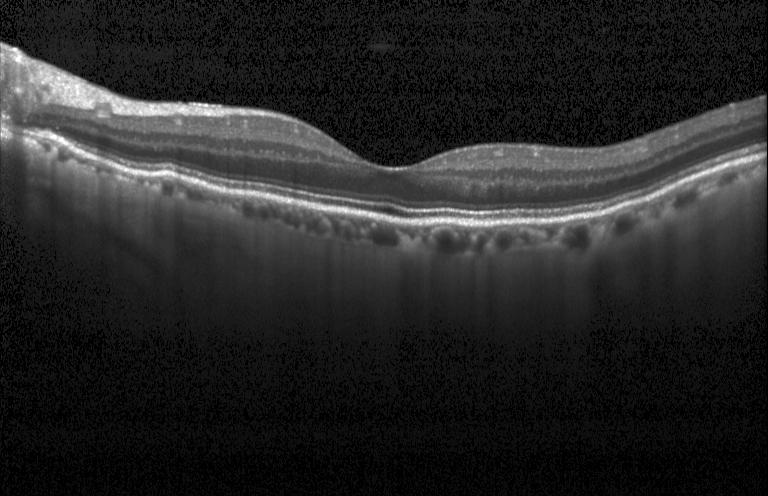 Acquired on a Heidelberg Spectralis, OCT B-scan, spectral-domain optical coherence tomography, centered on the fovea
OCT finding: no choroidal neovascularization, no diabetic macular edema, and no drusen.